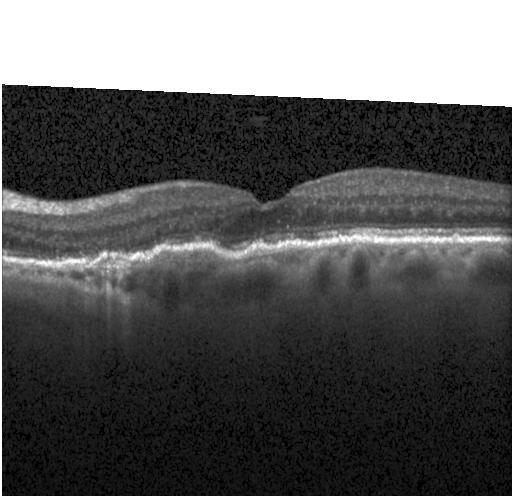 OCT B-scan
Assessment: a choroidal neovascular membrane.